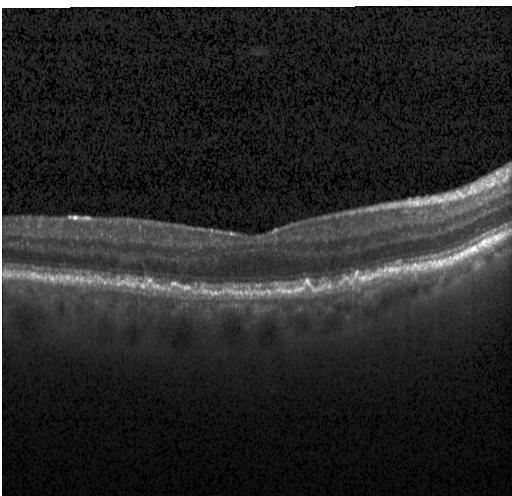

Centered on the fovea. Instrument: Heidelberg Spectralis. SD-OCT. Optical coherence tomography scan
Sub-RPE drusenoid deposits.